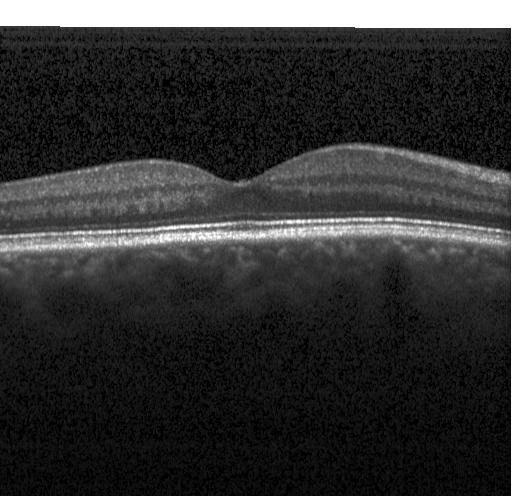

OCT B-scan showing no choroidal neovascularization, no diabetic macular edema, and no drusen.